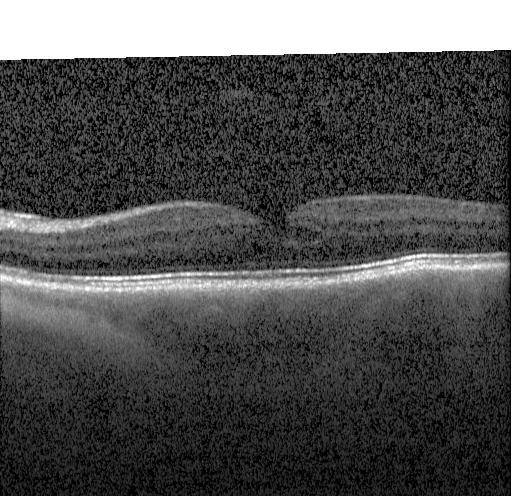
Retinal OCT B-scan; SD-OCT.
The scan shows diabetic macular edema.